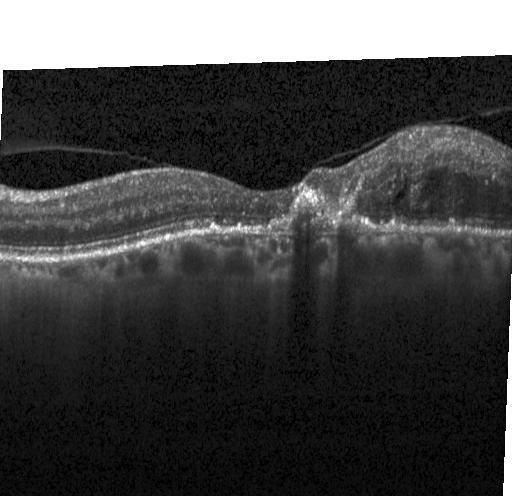 Impression: a choroidal neovascular membrane.